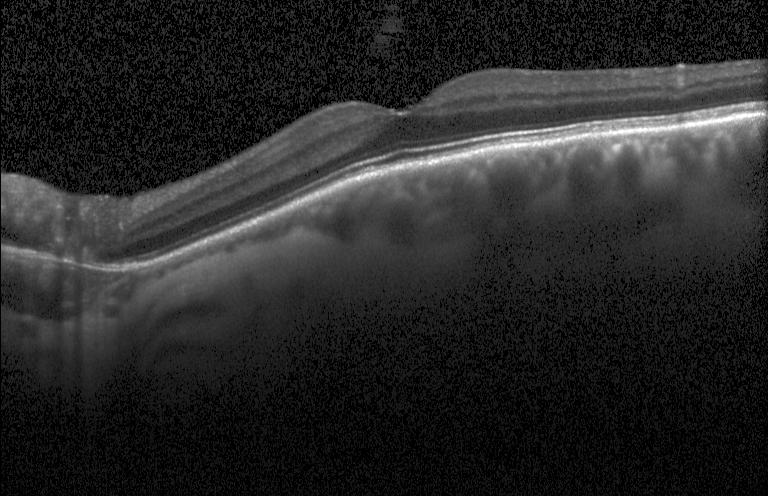 Instrument: Heidelberg Spectralis · OCT line scan — Finding: no choroidal neovascularization, no diabetic macular edema, and no drusen.